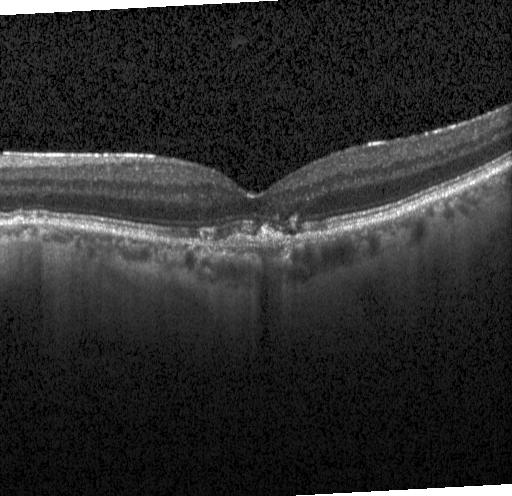 Finding: CNV.